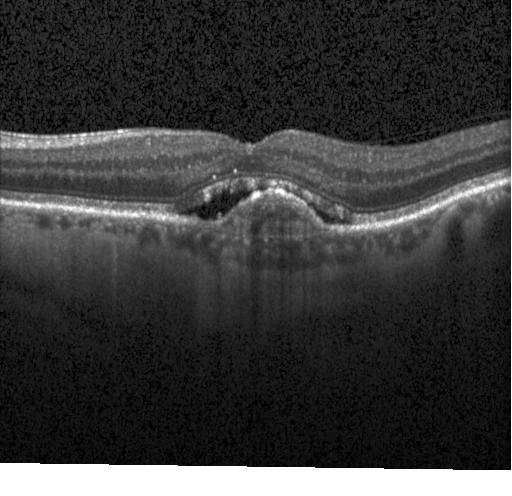 Retinal OCT cross-section. Spectral-domain optical coherence tomography. Assessment: a choroidal neovascular membrane.